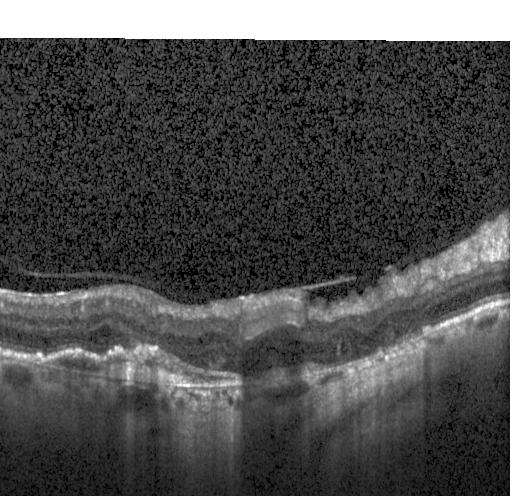

Assessment: a choroidal neovascular membrane.